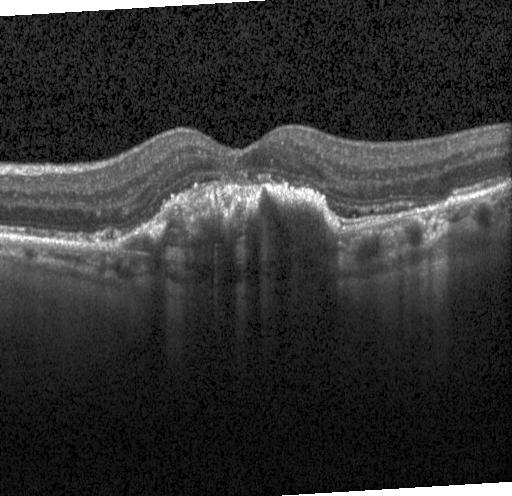 OCT B-scan.
A choroidal neovascular membrane.